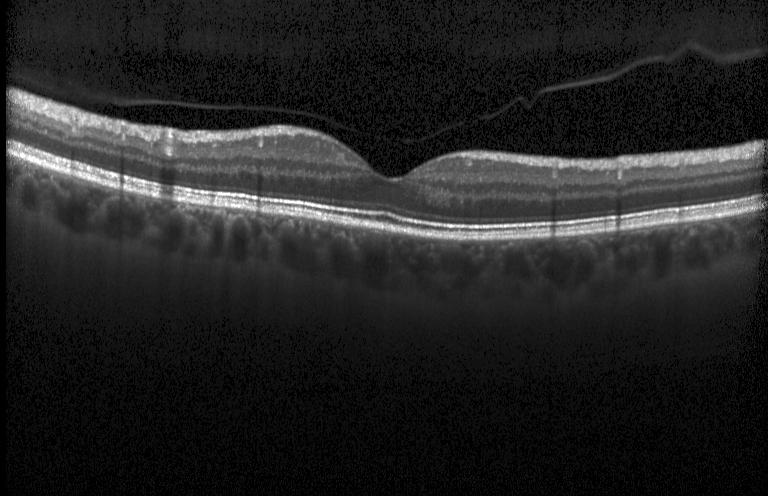 Retinal OCT cross-section; horizontal scan through the fovea; Heidelberg Spectralis OCT system; spectral-domain OCT.
Diagnosis: no CNV, DME, or drusen.